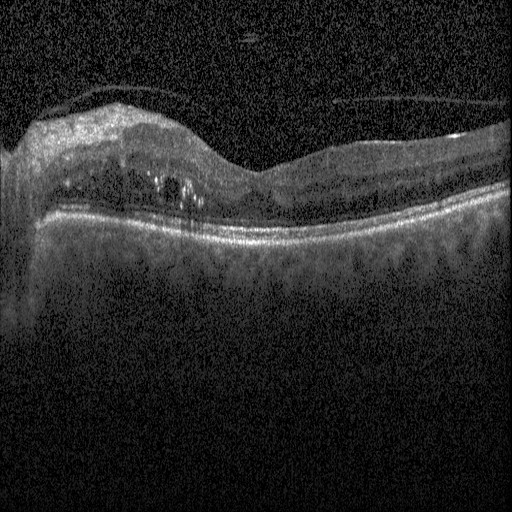

OCT B-scan — DME.